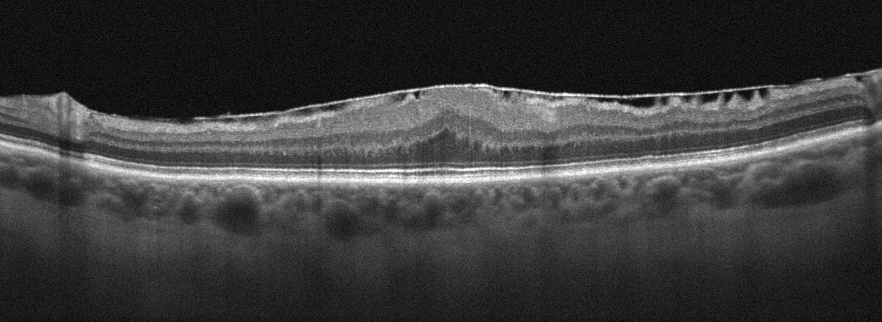
OS; retinal OCT cross-section.
Diagnosis: ERM.